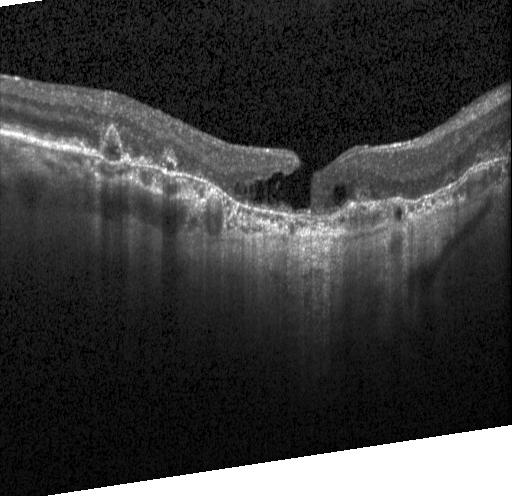
Centered on the fovea · acquired on a Heidelberg Spectralis · spectral-domain optical coherence tomography · optical coherence tomography B-scan.
Choroidal neovascularization (CNV).